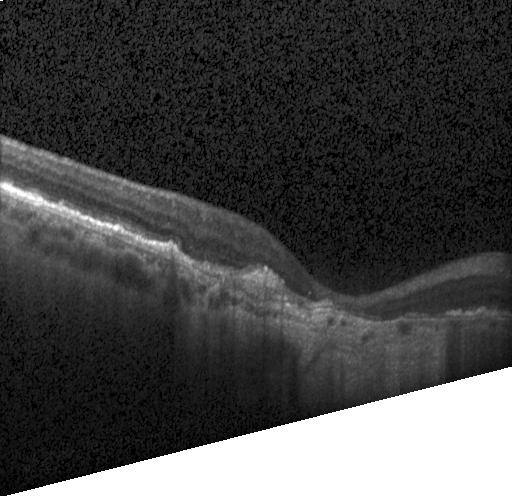 OCT scan showing a choroidal neovascular membrane.